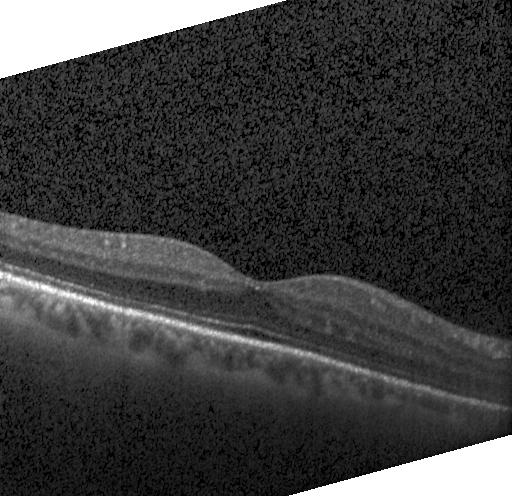 Macular scan. Optical coherence tomography scan. Heidelberg Spectralis OCT system.
Macular OCT: neither choroidal neovascularization, diabetic macular edema, nor drusen.